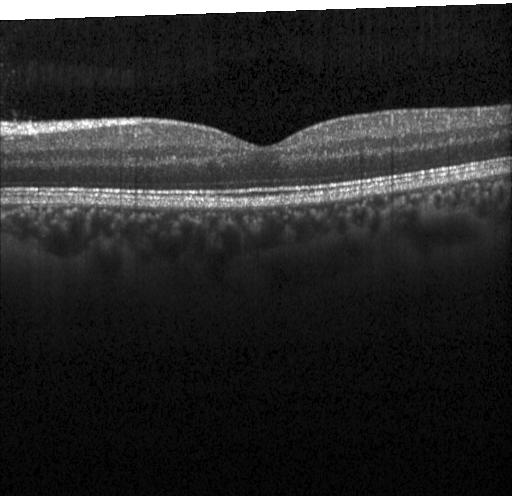

OCT B-scan.
Assessment: no choroidal neovascularization, diabetic macular edema, or drusen.